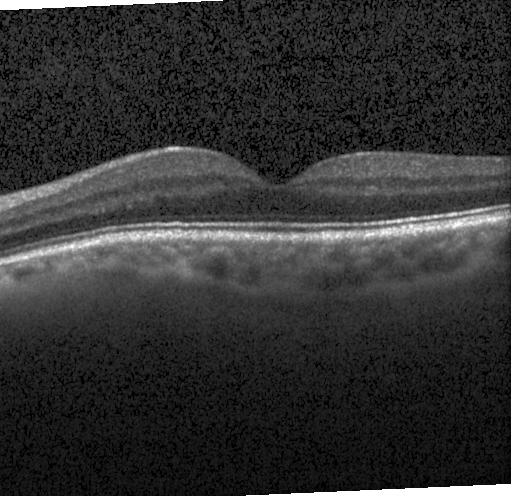

Spectral-domain optical coherence tomography; OCT B-scan; through the macula.
Impression: no CNV, DME, or drusen.